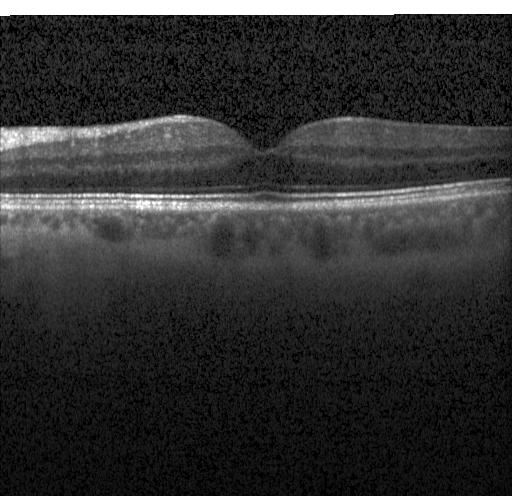
OCT B-scan. This B-scan demonstrates no evidence of choroidal neovascularization, diabetic macular edema, or drusen.